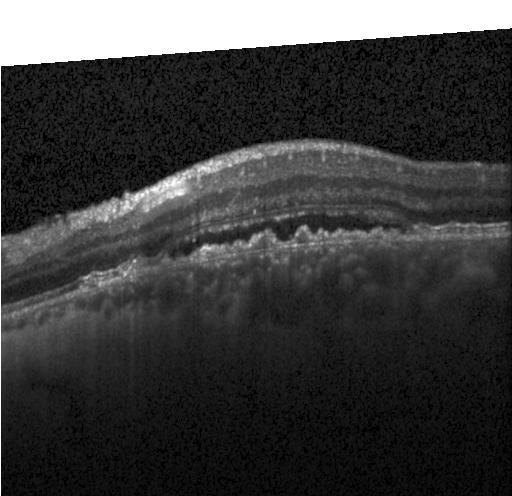
OCT finding: a choroidal neovascular membrane.